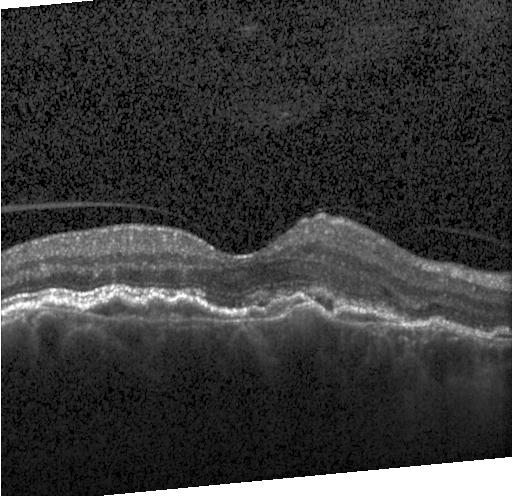

Impression: a choroidal neovascular membrane.